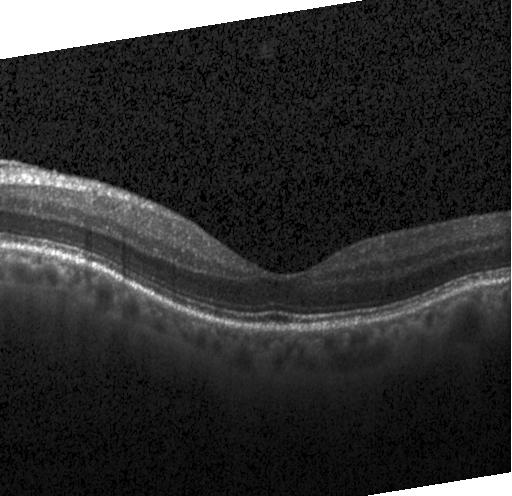
Spectral-domain optical coherence tomography · retinal OCT B-scan · fovea-centered · Heidelberg Spectralis
Finding: no choroidal neovascularization, diabetic macular edema, or drusen.